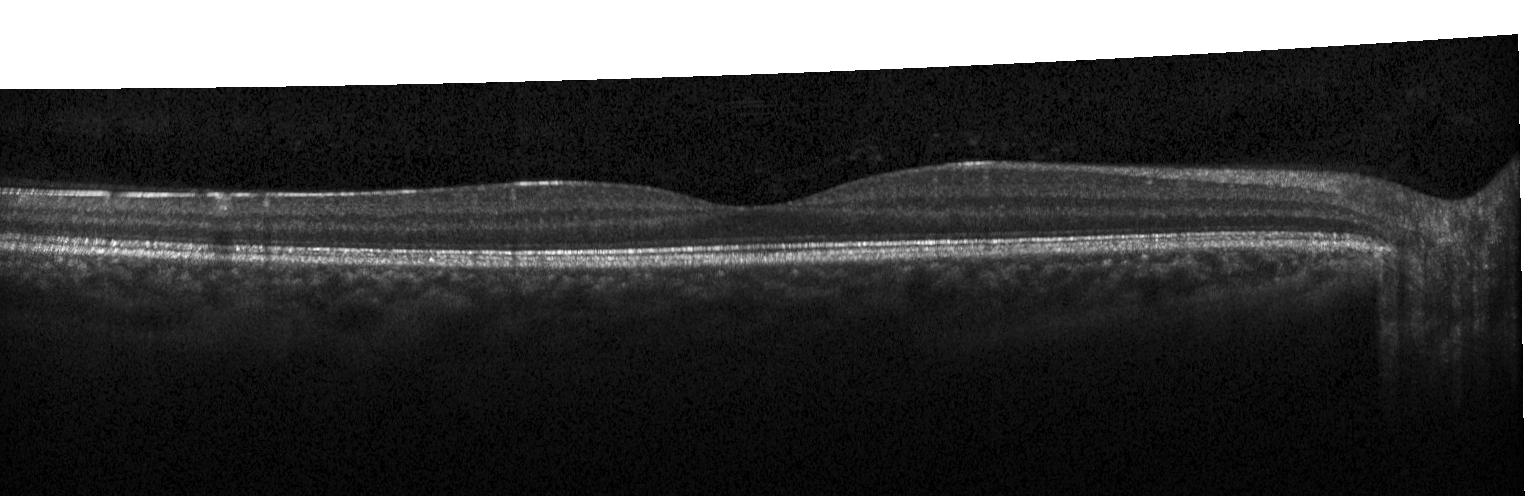
Through the macula; Heidelberg Spectralis; optical coherence tomography B-scan
The scan shows no choroidal neovascularization, no diabetic macular edema, and no drusen.